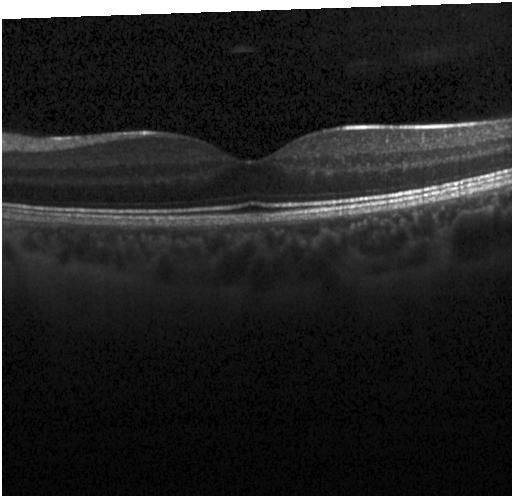

OCT line scan. Dx: no choroidal neovascularization, diabetic macular edema, or drusen.